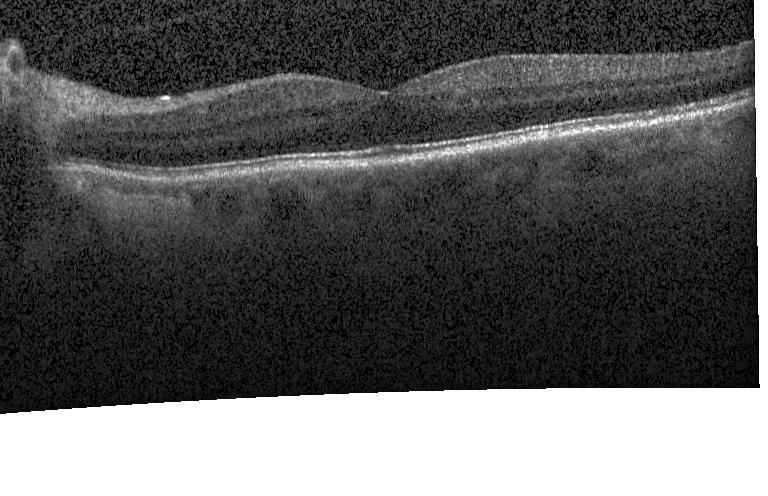

OCT line scan · centered on the fovea · instrument: Heidelberg Spectralis · SD-OCT.
Diagnosis: no evidence of choroidal neovascularization, diabetic macular edema, or drusen.